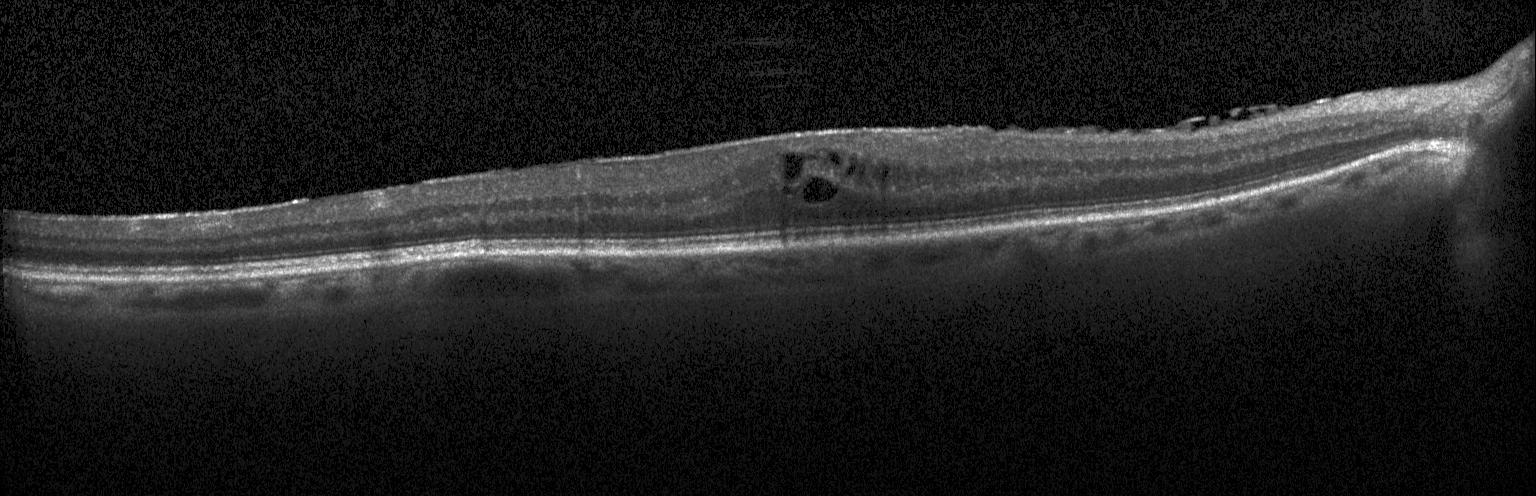

Impression: DME.